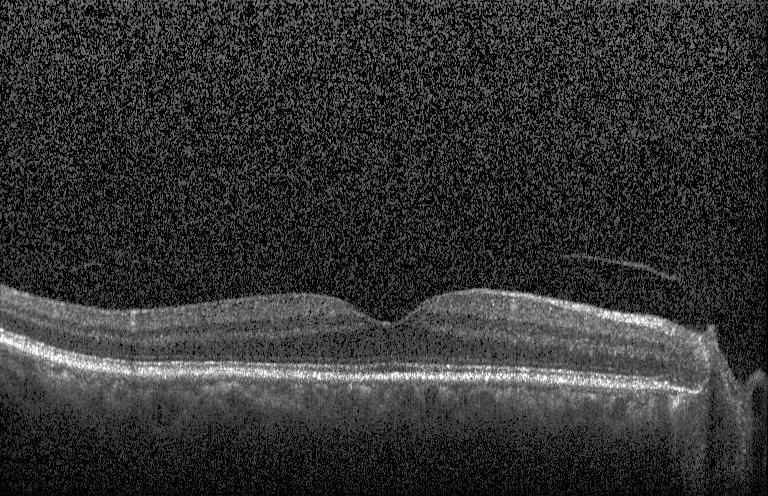
Neither CNV, DME, nor drusen.